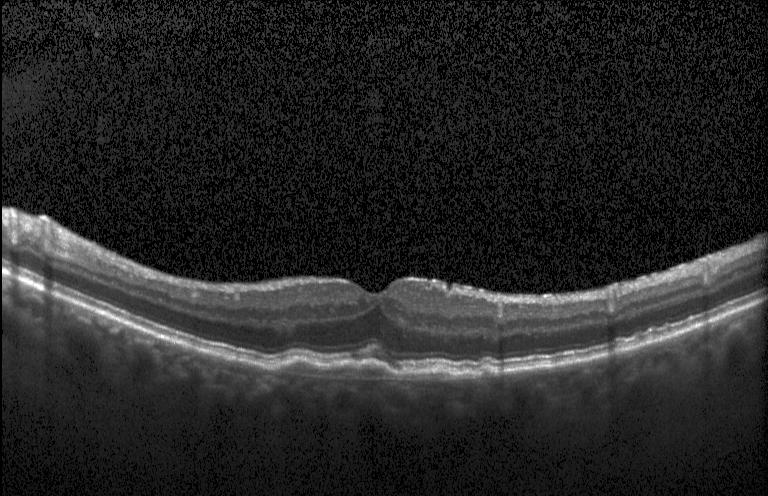 SD-OCT · optical coherence tomography B-scan — Diagnosis: a choroidal neovascular membrane.